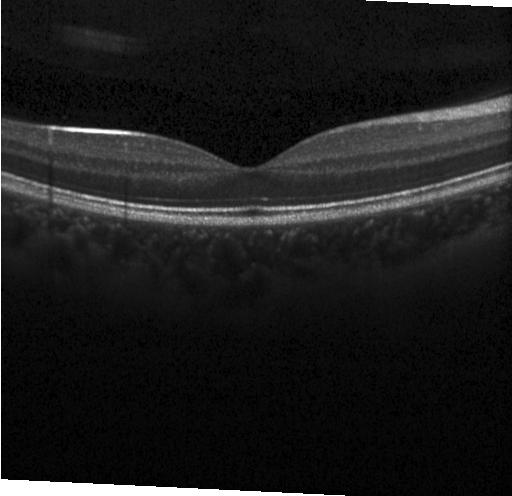

OCT B-scan · SD-OCT · Heidelberg Spectralis · fovea-centered. Assessment: no choroidal neovascularization, no diabetic macular edema, and no drusen.